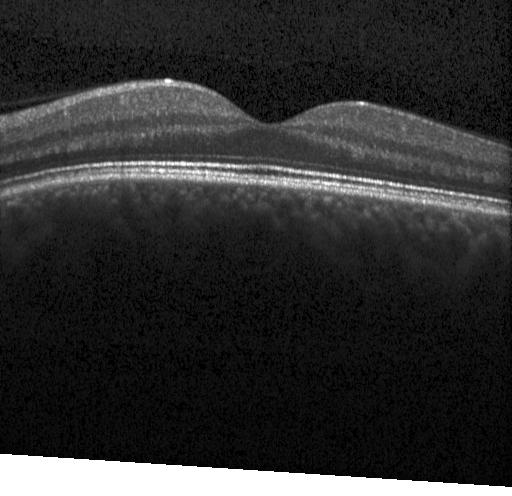
Heidelberg Spectralis; optical coherence tomography B-scan.
Finding: no CNV, DME, or drusen.